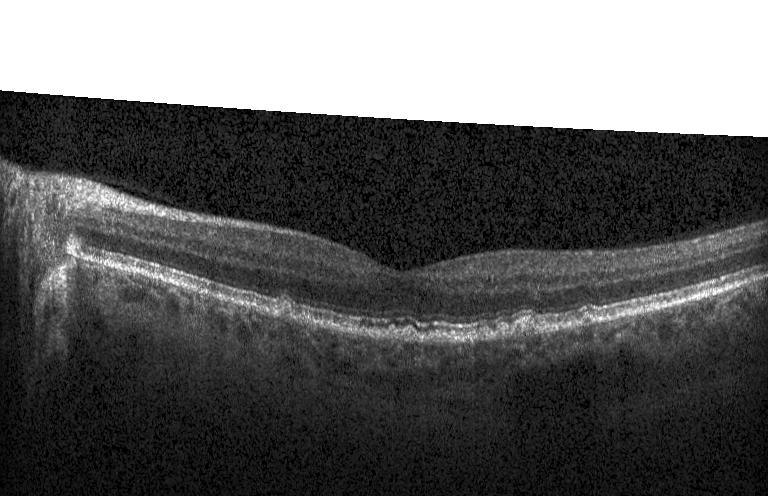
Acquired on a Heidelberg Spectralis · optical coherence tomography B-scan
Diagnosis: drusen.